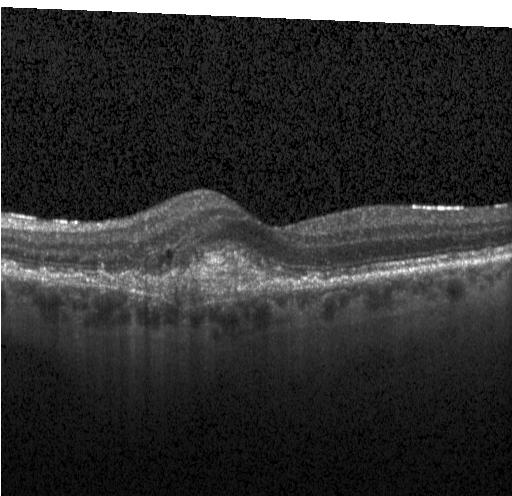 Dx: CNV.